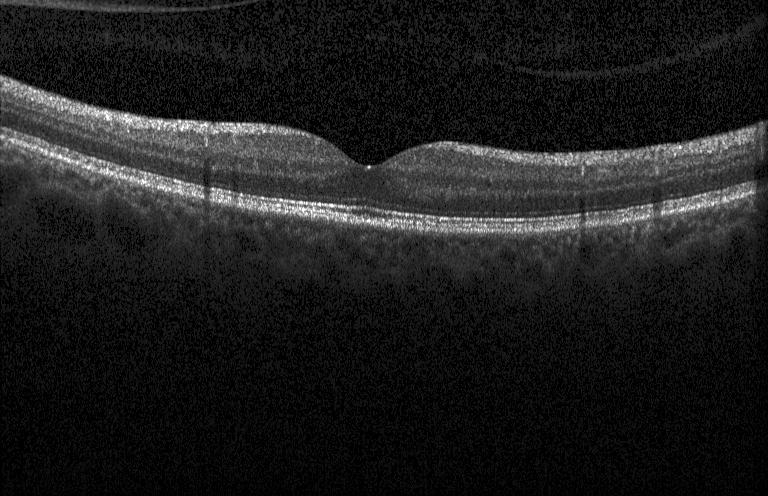
Optical coherence tomography scan
Impression: no choroidal neovascularization, diabetic macular edema, or drusen.